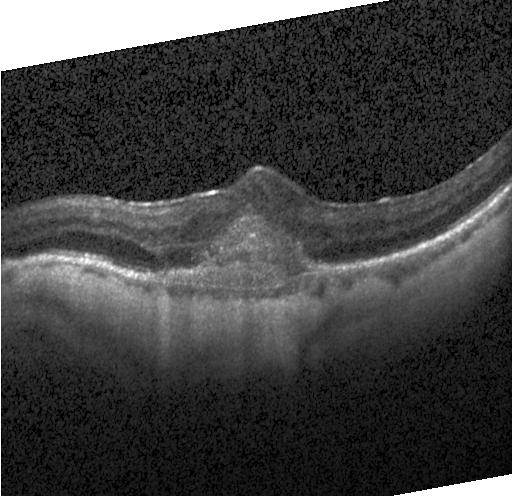

Finding: choroidal neovascularization (CNV).